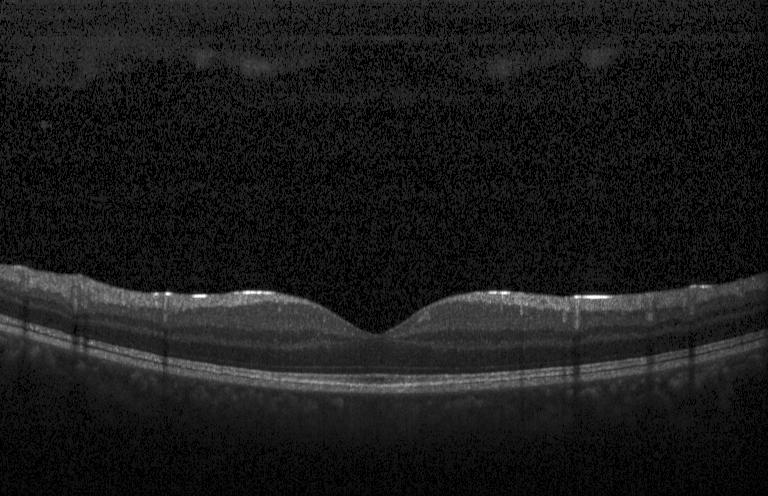
Through the macula · retinal OCT cross-section — Finding: no evidence of CNV, DME, or drusen.